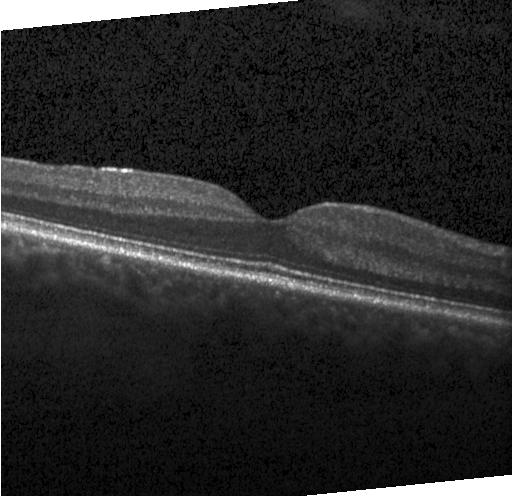 Optical coherence tomography scan · Heidelberg Spectralis OCT system · spectral-domain optical coherence tomography.
The scan shows neither choroidal neovascularization, diabetic macular edema, nor drusen.